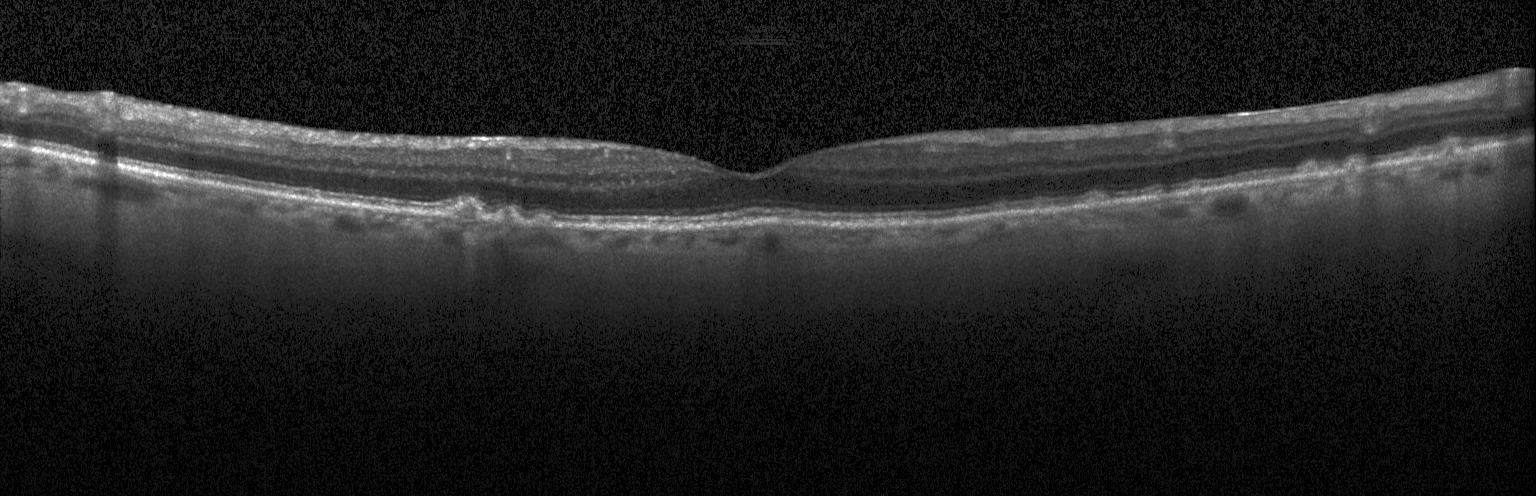
Macular OCT demonstrating multiple drusen.